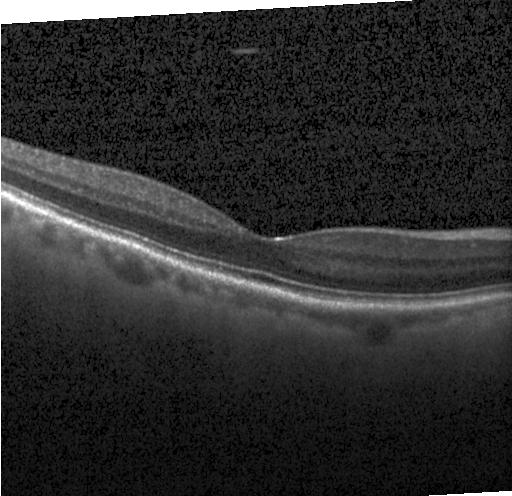

Optical coherence tomography scan — The scan shows no choroidal neovascularization, no diabetic macular edema, and no drusen.